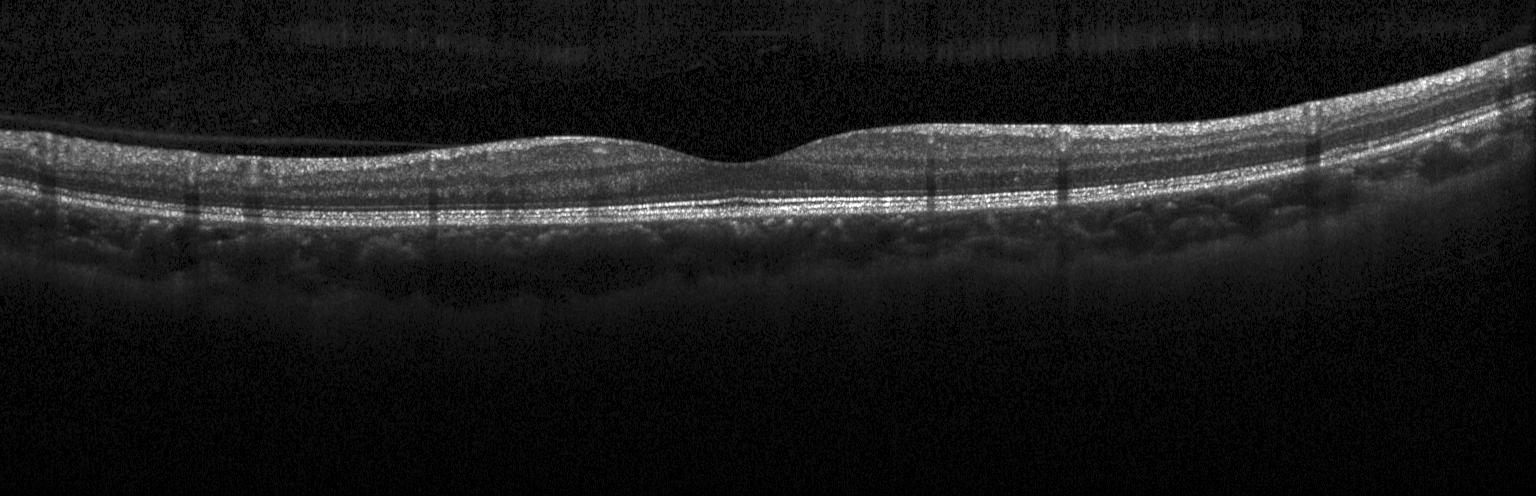
Retinal OCT cross-section showing no CNV, DME, or drusen.